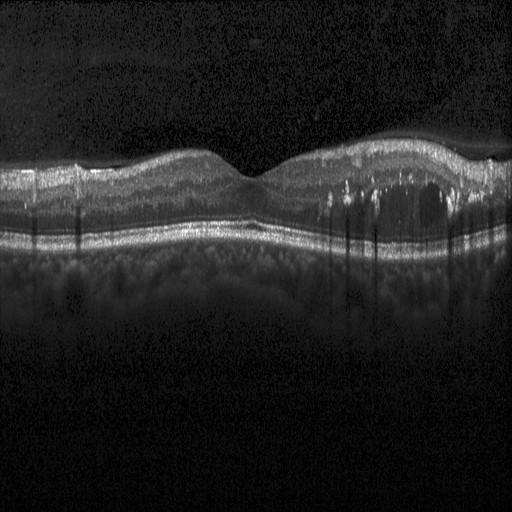

Optical coherence tomography scan. The scan shows DME.